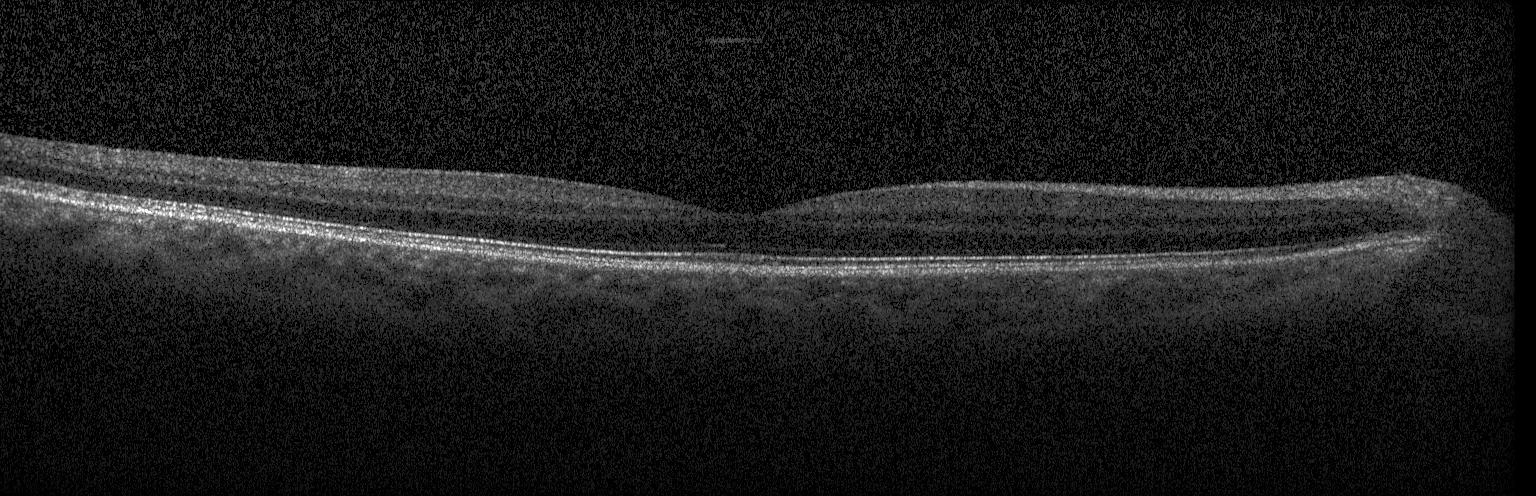

Horizontal scan through the fovea · Heidelberg Spectralis OCT system · OCT B-scan · SD-OCT
Impression: neither choroidal neovascularization, diabetic macular edema, nor drusen.